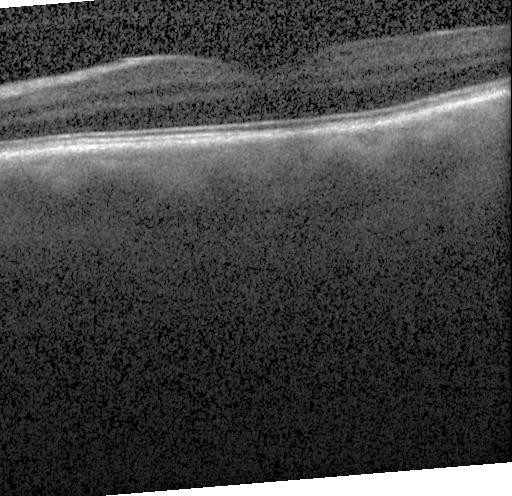
Fovea-centered · retinal OCT cross-section.
OCT finding: neither choroidal neovascularization, diabetic macular edema, nor drusen.